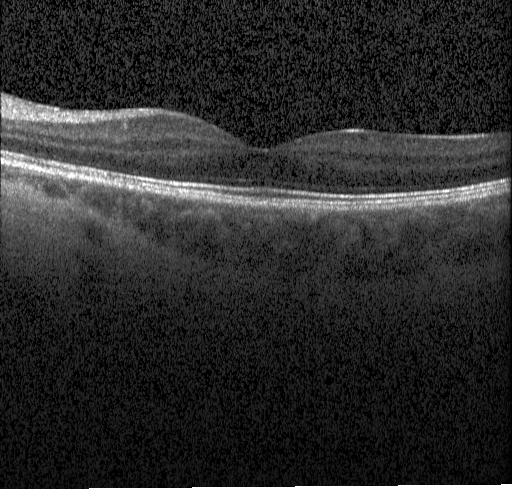

Optical coherence tomography B-scan; spectral-domain OCT; centered on the fovea.
OCT finding: no evidence of choroidal neovascularization, diabetic macular edema, or drusen.